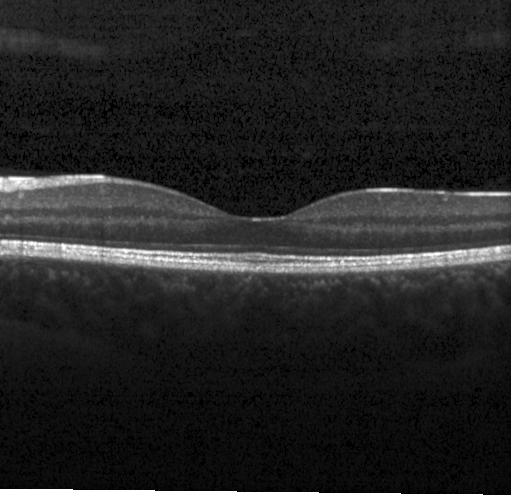

Optical coherence tomography B-scan, acquired on a Heidelberg Spectralis, spectral-domain OCT, centered on the fovea. Dx: no CNV, DME, or drusen.